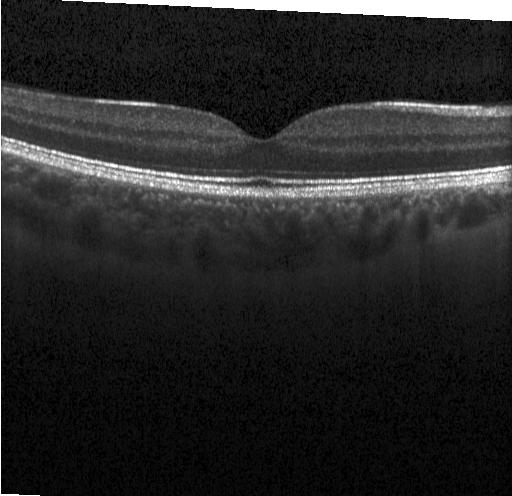

Spectral-domain OCT; retinal OCT cross-section; fovea-centered — Finding: no CNV, no DME, and no drusen.